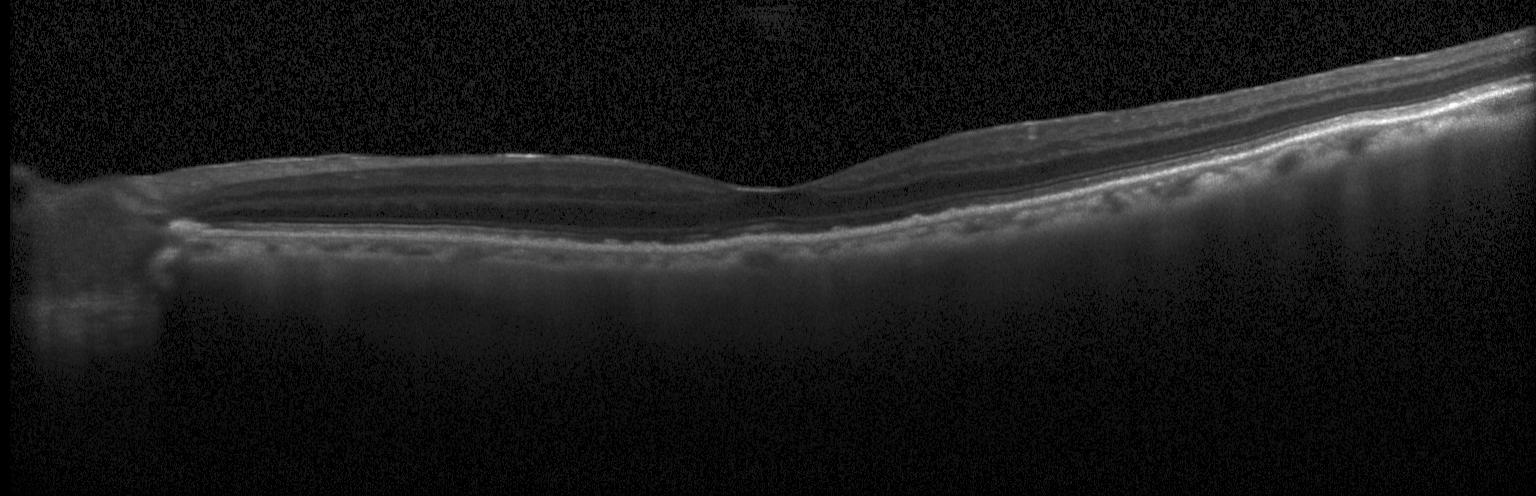

Retinal OCT cross-section showing sub-RPE drusenoid deposits.